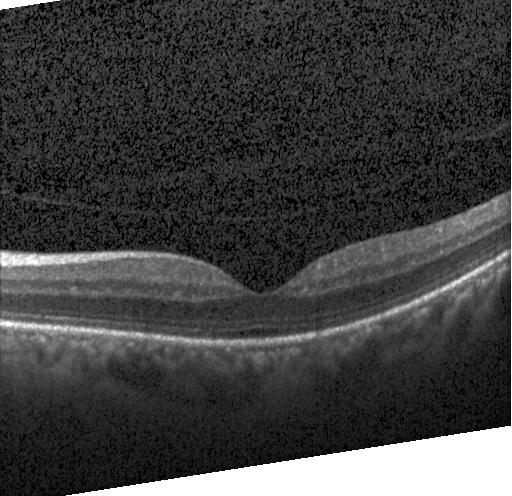

SD-OCT. Optical coherence tomography B-scan. Horizontal scan through the fovea. Macular OCT: neither choroidal neovascularization, diabetic macular edema, nor drusen.